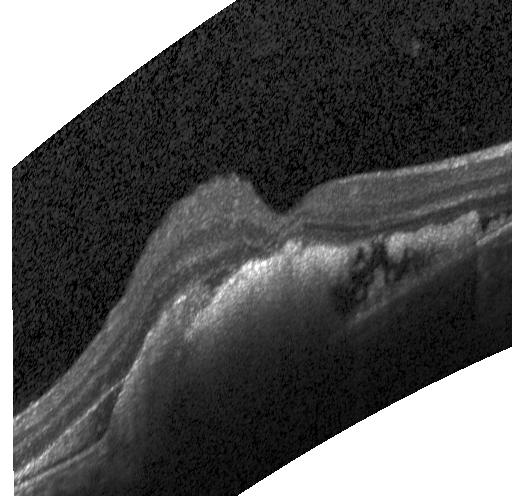 Macular OCT demonstrating choroidal neovascularization (CNV).